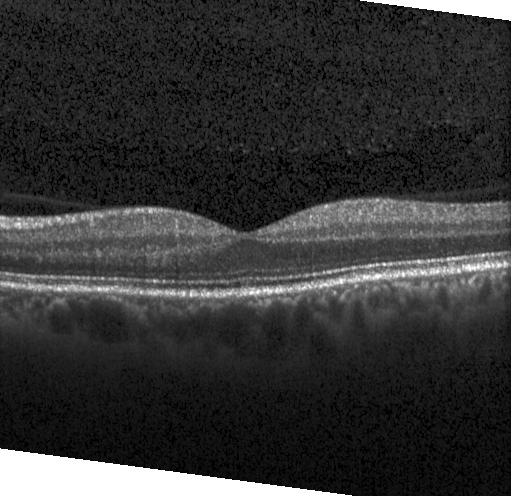 Diagnosis: neither CNV, DME, nor drusen.